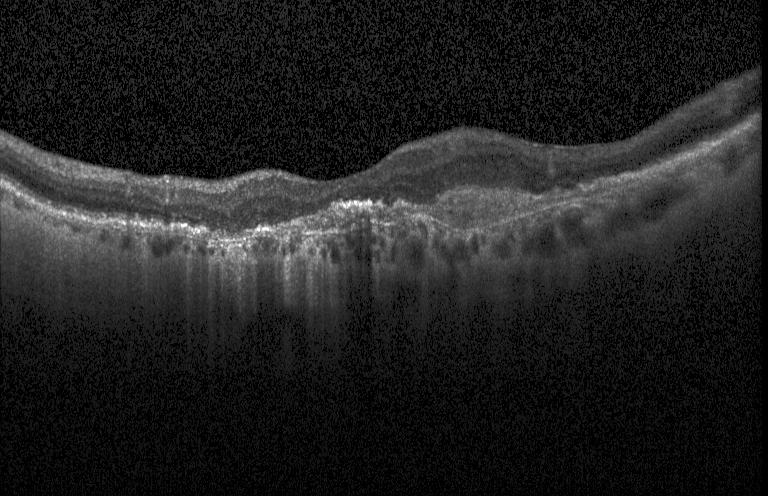
Retinal OCT cross-section. Macular OCT: choroidal neovascularization.